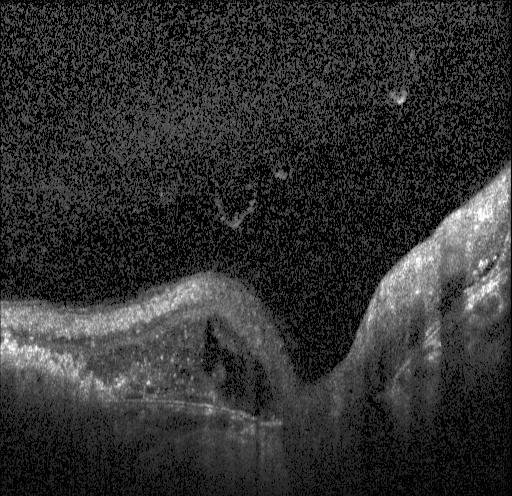
Finding: choroidal neovascularization (CNV).